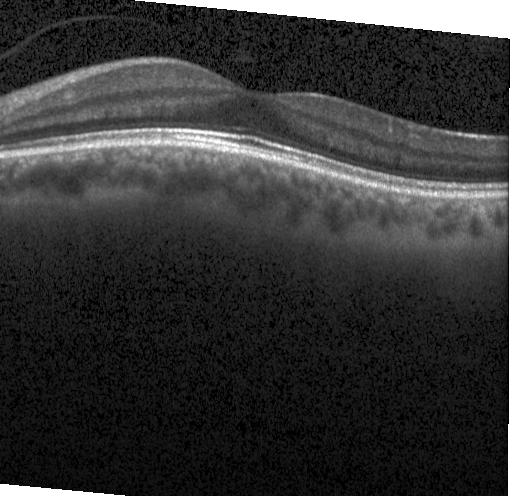
Optical coherence tomography B-scan. Instrument: Heidelberg Spectralis. Fovea-centered — Diagnosis: no choroidal neovascularization, diabetic macular edema, or drusen.